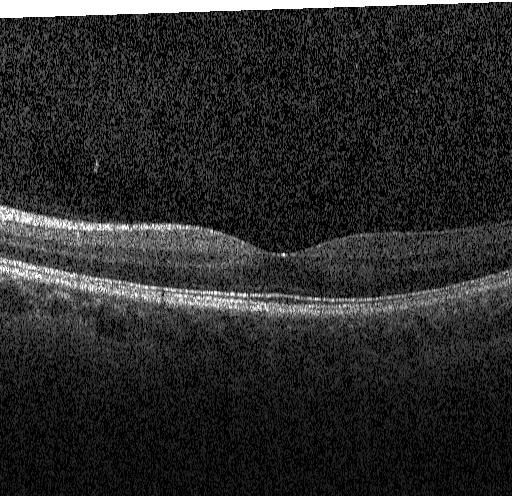 OCT B-scan showing neither choroidal neovascularization, diabetic macular edema, nor drusen.